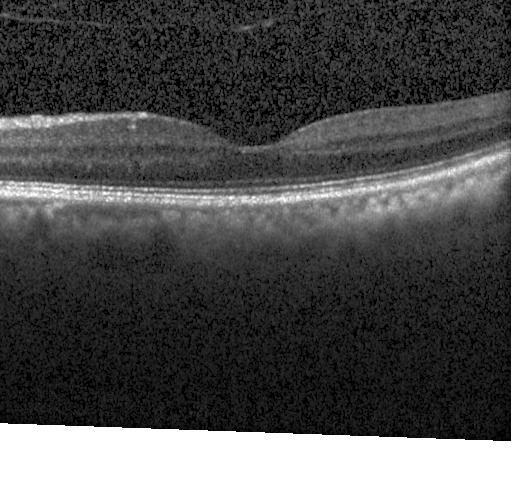 Impression: no CNV, DME, or drusen.